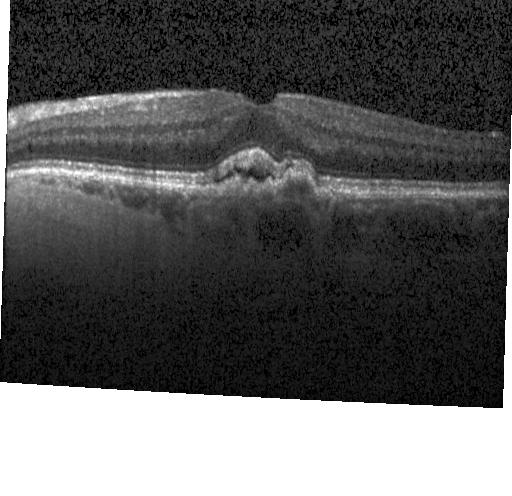 Macular scan, Heidelberg Spectralis OCT system, spectral-domain OCT, retinal OCT B-scan. Assessment: a choroidal neovascular membrane.